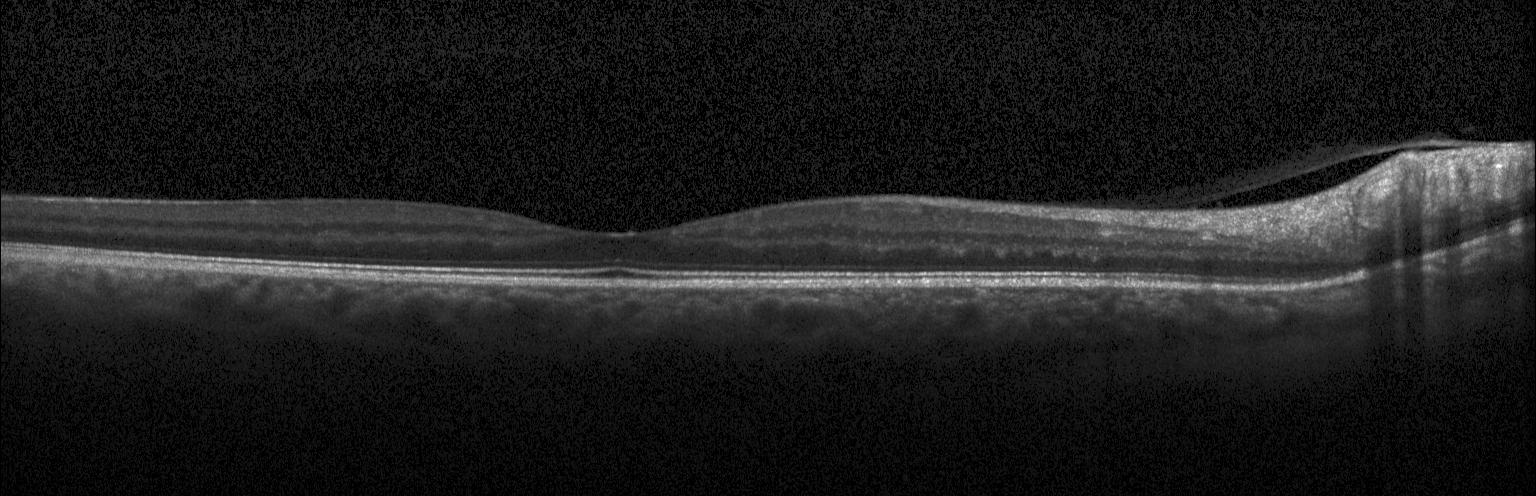 OCT finding: no choroidal neovascularization, diabetic macular edema, or drusen.